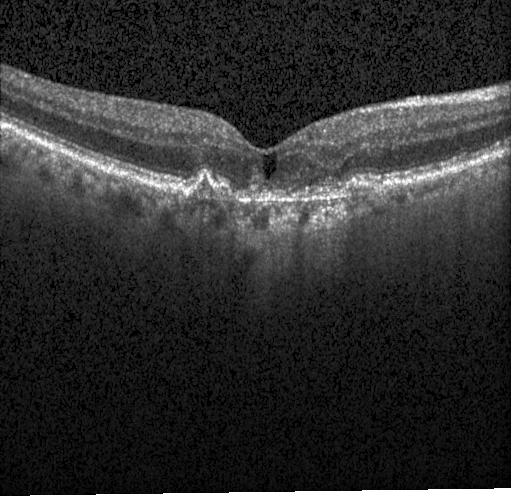 Retinal OCT cross-section. Impression: a choroidal neovascular membrane.